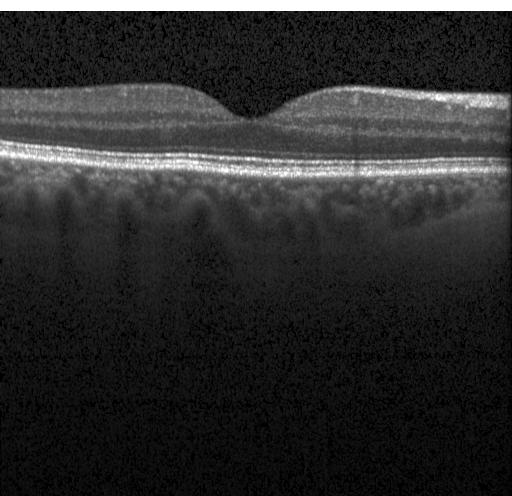 Dx: no evidence of choroidal neovascularization, diabetic macular edema, or drusen.